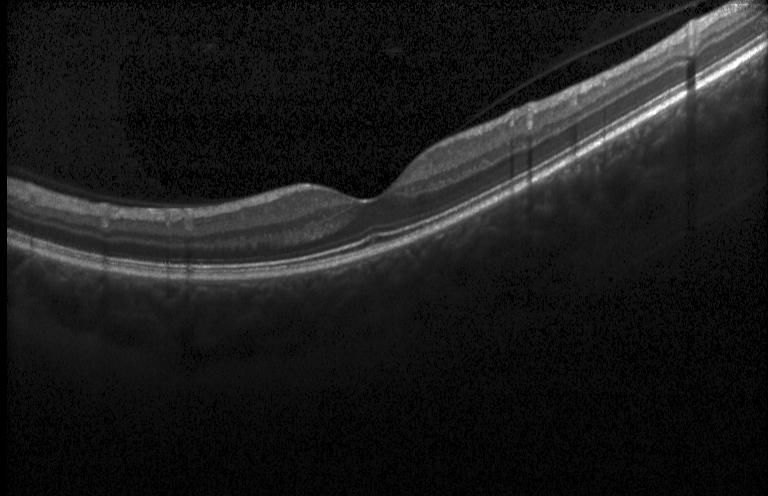
OCT B-scan showing no evidence of choroidal neovascularization, diabetic macular edema, or drusen.